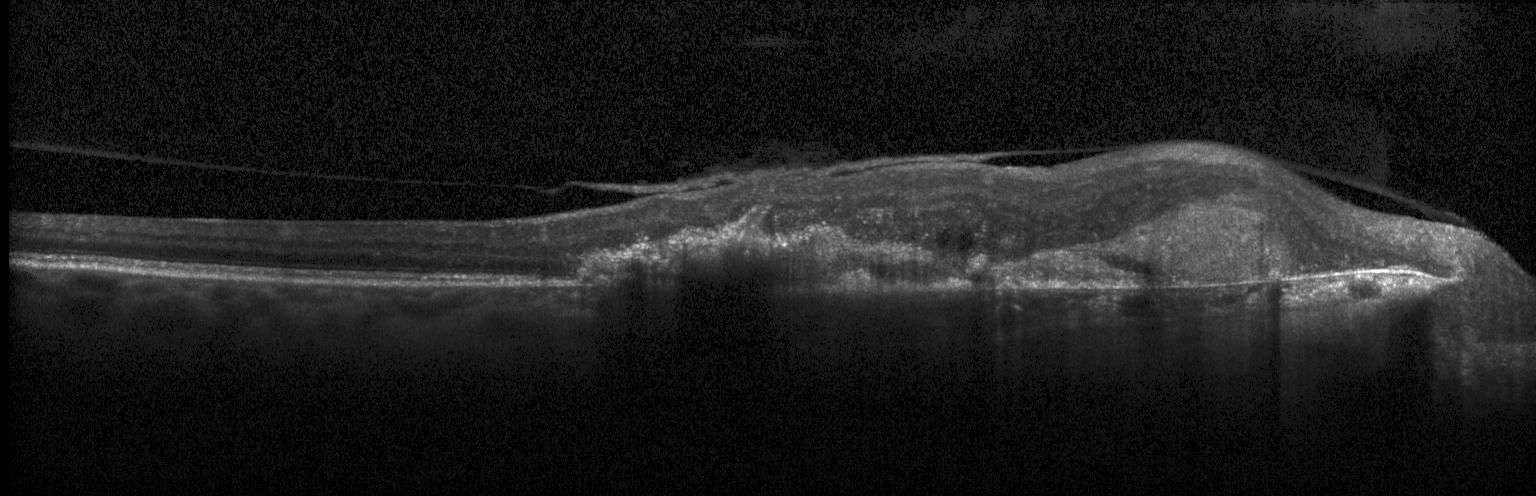
Spectral-domain OCT B-scan: choroidal neovascularization.